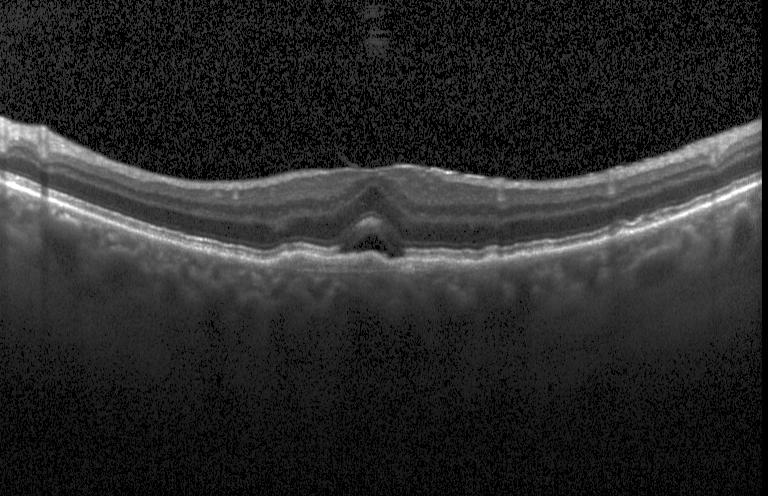

Optical coherence tomography scan. Heidelberg Spectralis. Dx: a choroidal neovascular membrane.